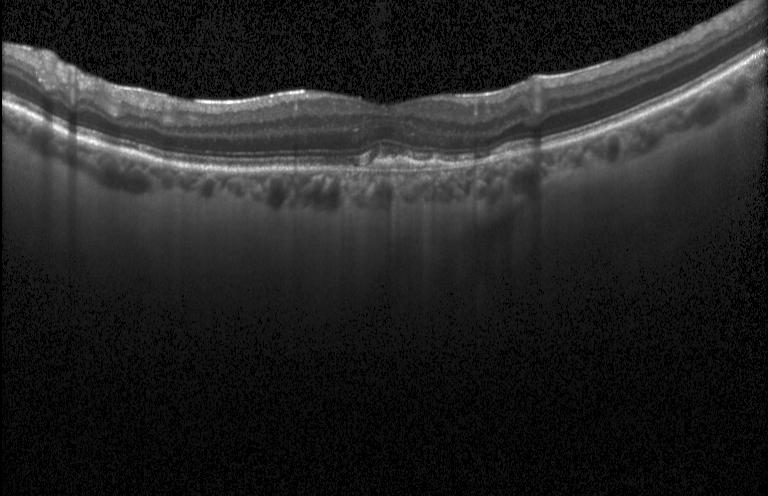

SD-OCT · retinal OCT B-scan · acquired on a Heidelberg Spectralis.
This B-scan demonstrates choroidal neovascularization (CNV).